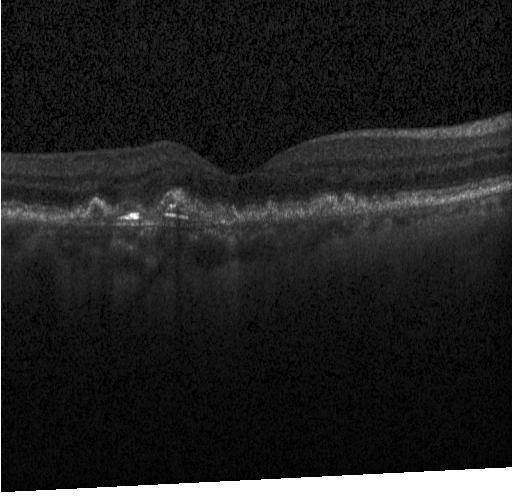

OCT B-scan showing a choroidal neovascular membrane.